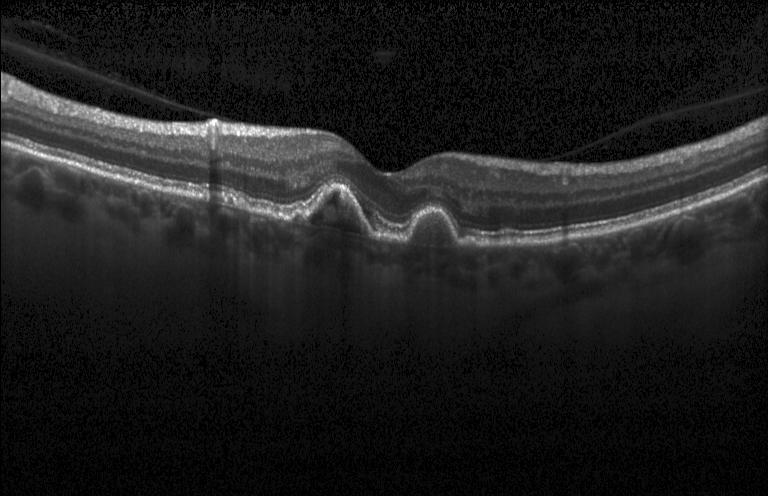

Through the macula · acquired on a Heidelberg Spectralis · optical coherence tomography B-scan. This B-scan demonstrates drusen.